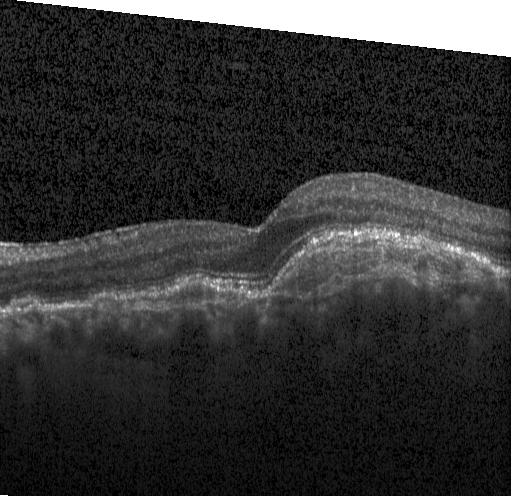

Finding: a choroidal neovascular membrane.